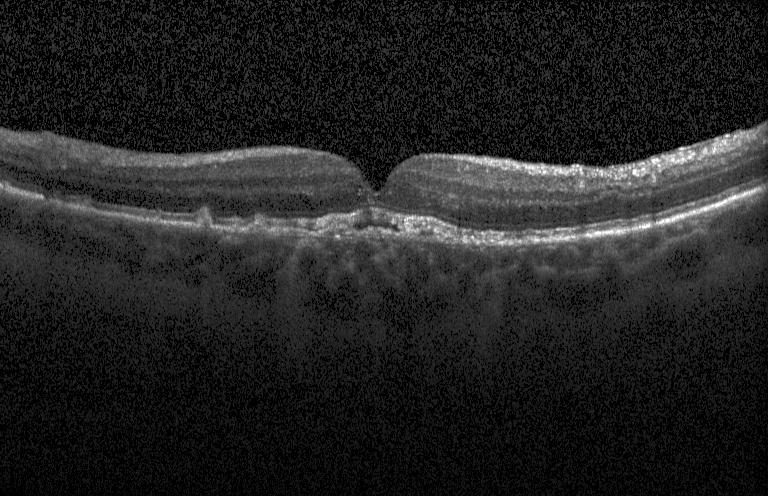

Finding: a choroidal neovascular membrane.